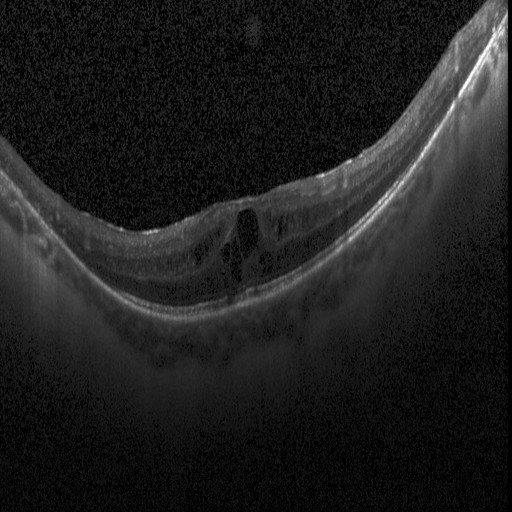 OCT B-scan.
Impression: DME.